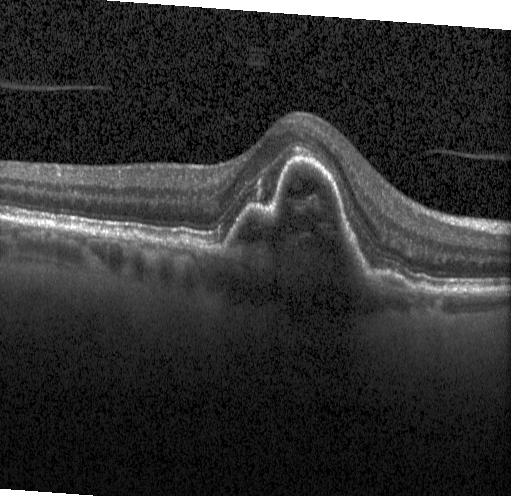 Optical coherence tomography B-scan — Finding: a choroidal neovascular membrane.